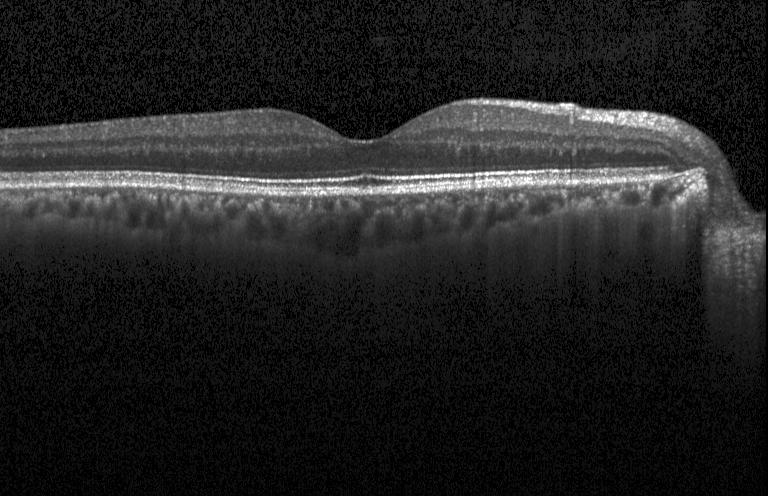

Through the macula; OCT B-scan; Heidelberg Spectralis OCT system. Finding: no CNV, DME, or drusen.